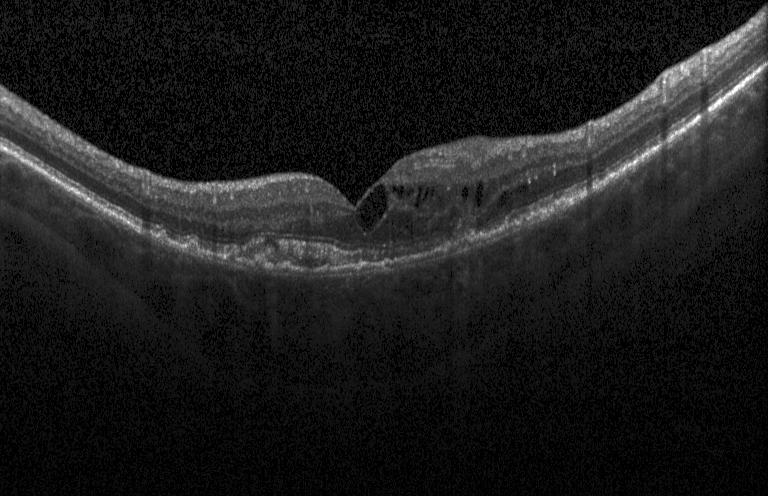 Fovea-centered · OCT line scan
Impression: choroidal neovascularization (CNV).